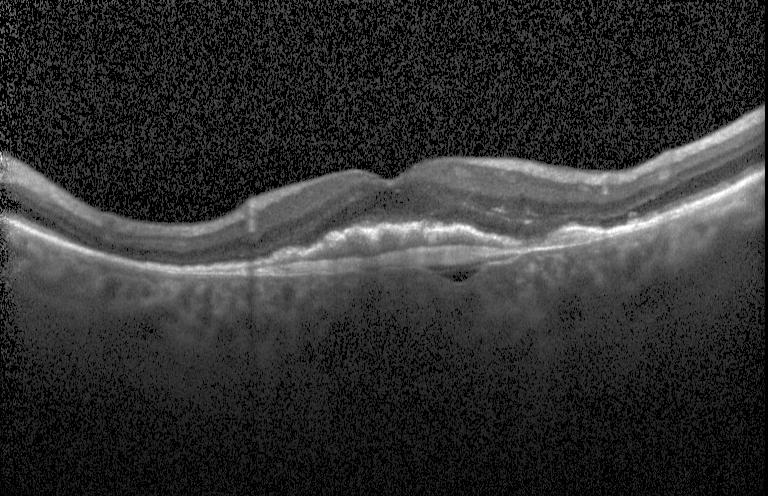 OCT B-scan — Impression: a choroidal neovascular membrane.